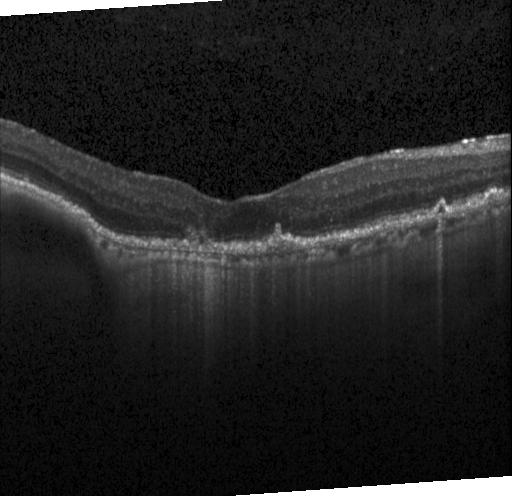 Retinal OCT cross-section showing choroidal neovascularization (CNV).